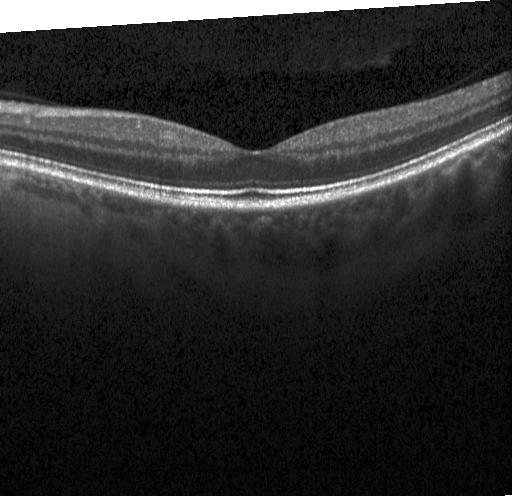
Retinal OCT B-scan, Heidelberg Spectralis
Impression: neither choroidal neovascularization, diabetic macular edema, nor drusen.